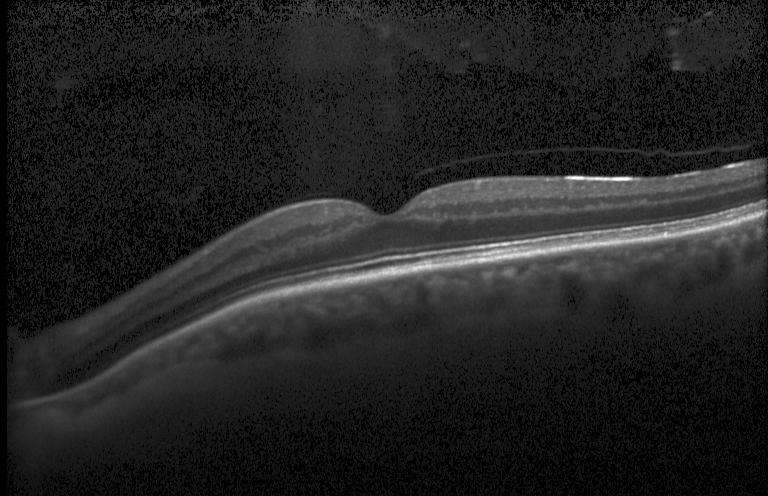 Spectral-domain optical coherence tomography. OCT B-scan. Horizontal scan through the fovea — Assessment: no evidence of CNV, DME, or drusen.